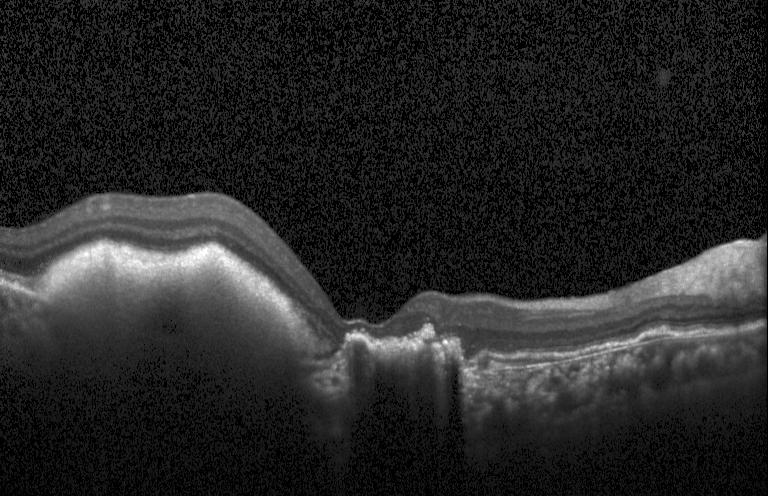
Acquired on a Heidelberg Spectralis. OCT line scan. SD-OCT — CNV.